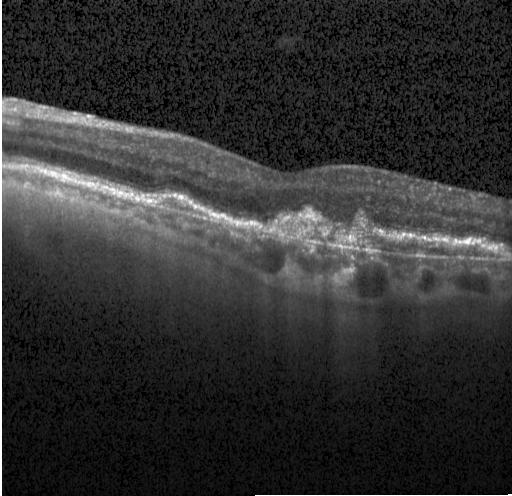

Horizontal scan through the fovea. Optical coherence tomography scan. Instrument: Heidelberg Spectralis. The scan shows CNV.